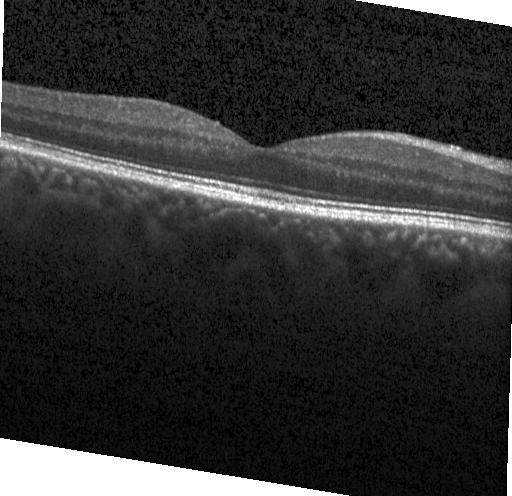

OCT scan showing no choroidal neovascularization, diabetic macular edema, or drusen.